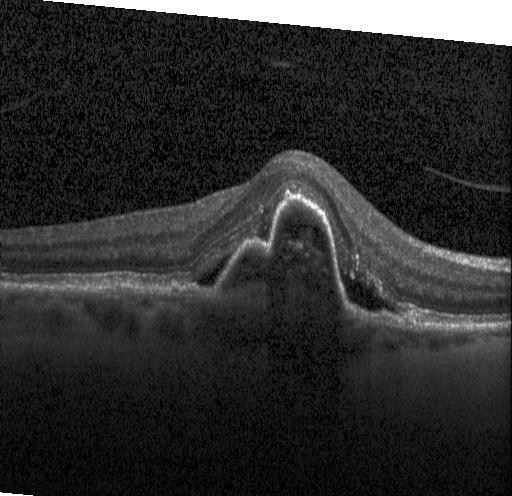
Retinal OCT B-scan
Finding: CNV.